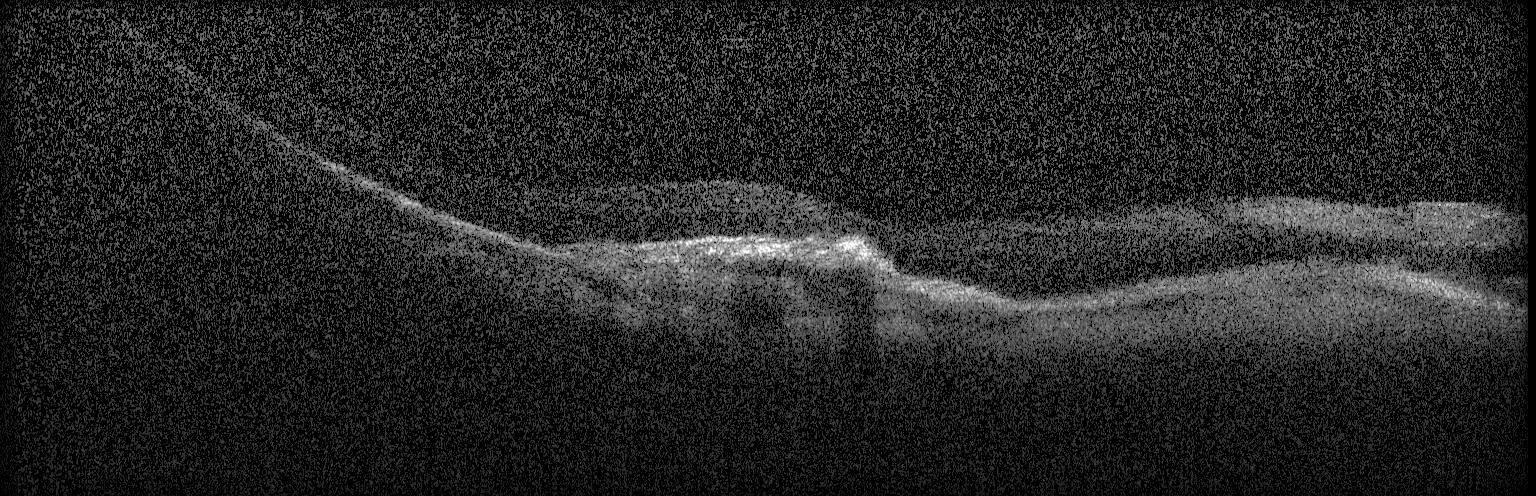

Heidelberg Spectralis OCT system, OCT B-scan, SD-OCT, fovea-centered.
Macular OCT: choroidal neovascularization.